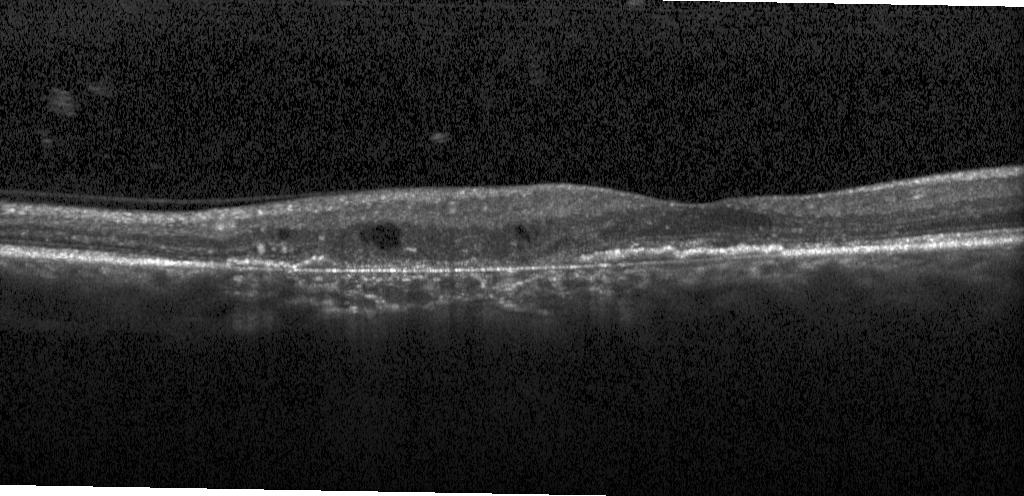

Macular scan, retinal OCT B-scan, spectral-domain OCT, acquired on a Heidelberg Spectralis — Impression: choroidal neovascularization.